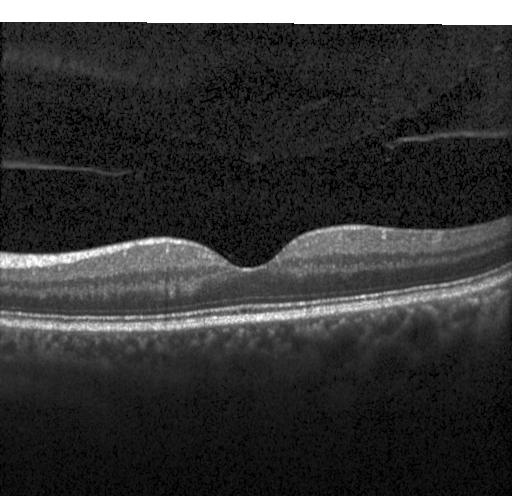
Spectral-domain OCT · optical coherence tomography scan · centered on the fovea
Finding: no CNV, DME, or drusen.